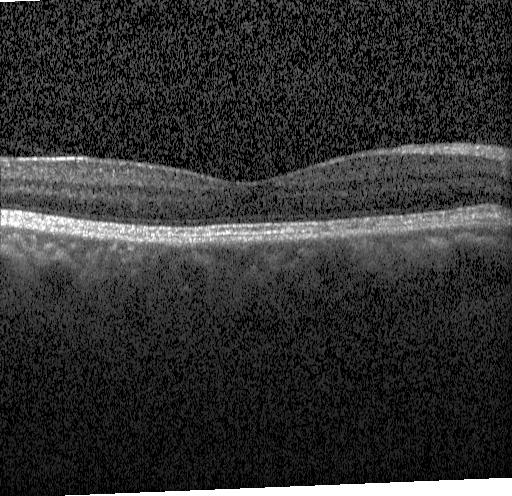 Spectral-domain OCT; OCT B-scan — Finding: neither choroidal neovascularization, diabetic macular edema, nor drusen.